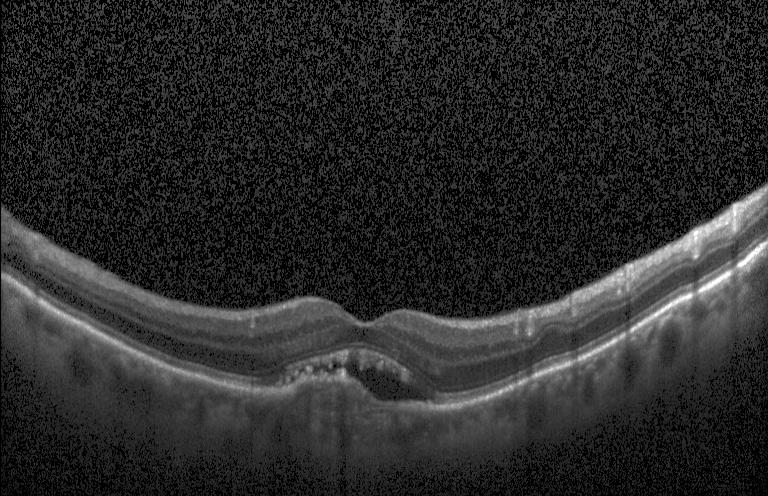

Horizontal scan through the fovea, OCT line scan
Impression: CNV.